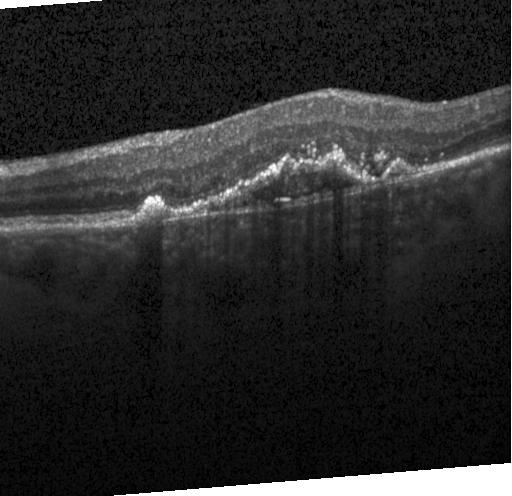

Instrument: Heidelberg Spectralis · optical coherence tomography scan — Impression: a choroidal neovascular membrane.